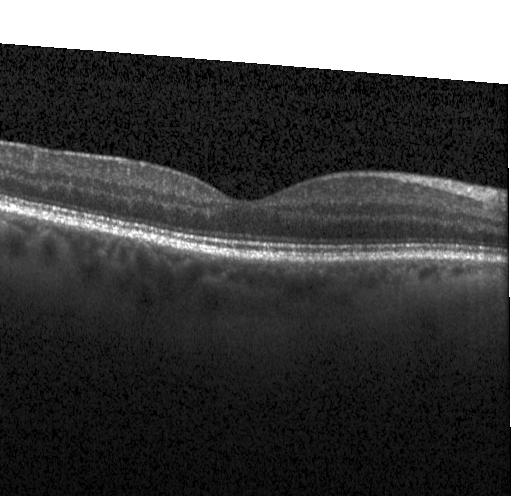
Heidelberg Spectralis. OCT B-scan. Spectral-domain OCT
This B-scan demonstrates no CNV, no DME, and no drusen.